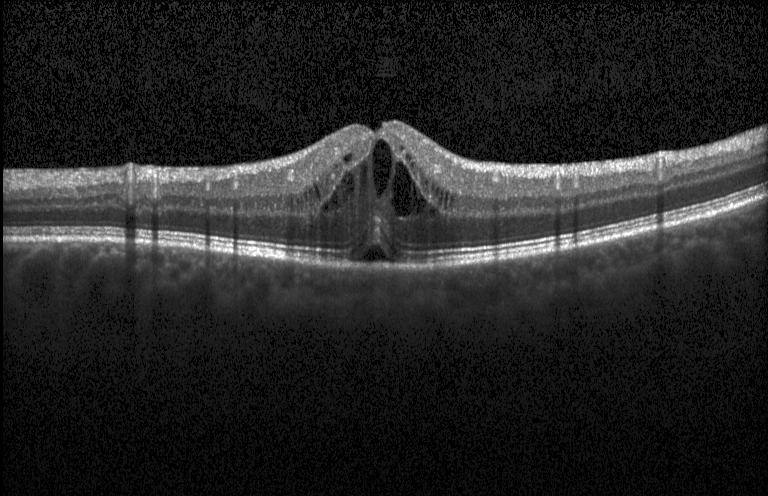

Spectral-domain optical coherence tomography · fovea-centered · retinal OCT cross-section · Heidelberg Spectralis — The scan shows diabetic macular edema (DME).